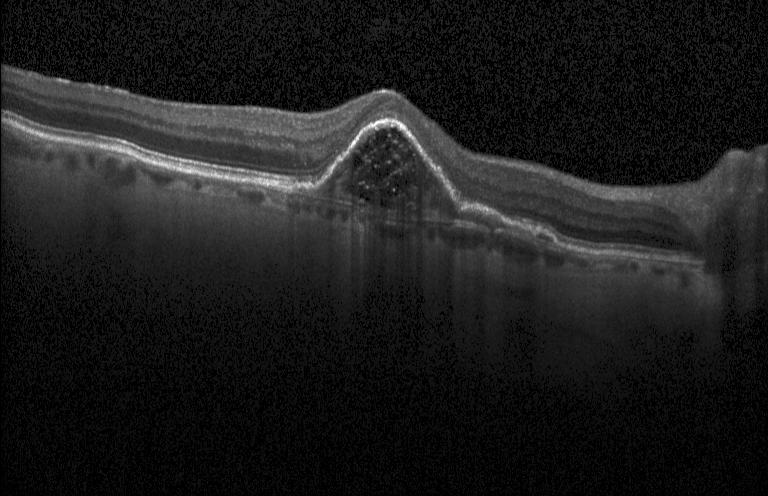 Retinal OCT B-scan. Macular OCT: a choroidal neovascular membrane.